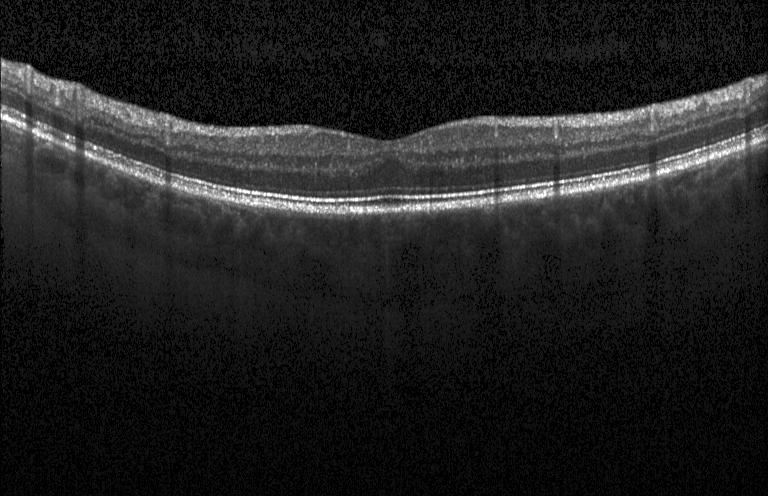

SD-OCT, retinal OCT B-scan
Finding: no choroidal neovascularization, diabetic macular edema, or drusen.